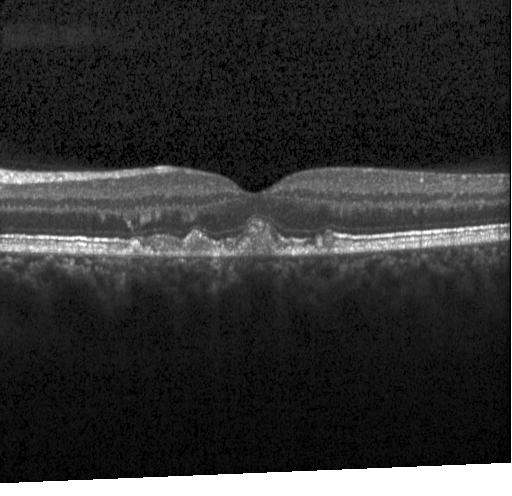

Retinal OCT cross-section · instrument: Heidelberg Spectralis · spectral-domain OCT · macular scan. Impression: multiple drusen.